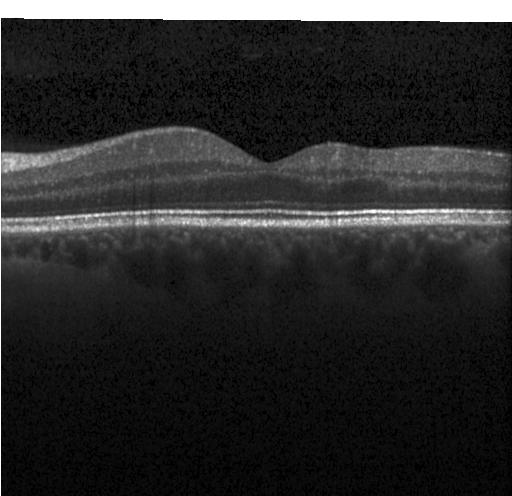 Dx: no choroidal neovascularization, no diabetic macular edema, and no drusen.